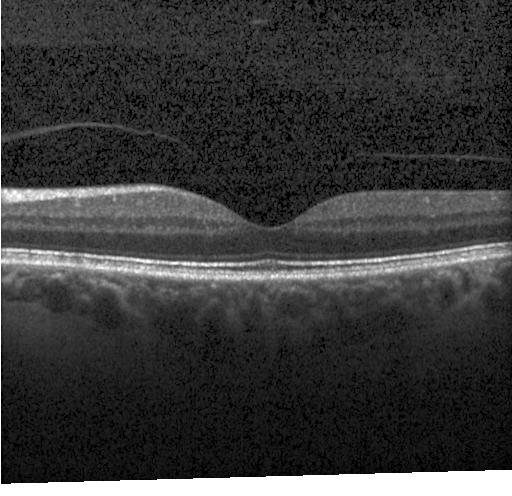
No choroidal neovascularization, diabetic macular edema, or drusen.